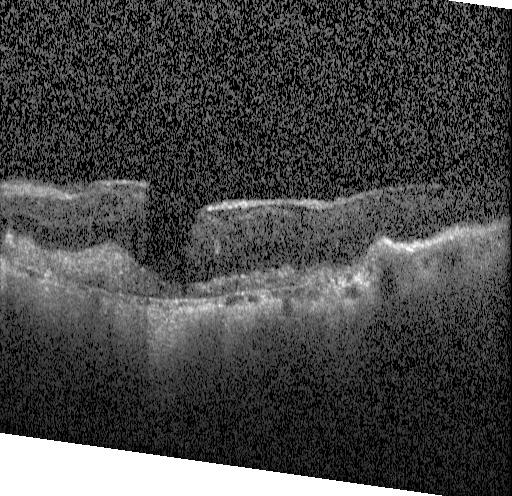
OCT B-scan · macular scan · spectral-domain optical coherence tomography · Heidelberg Spectralis.
Diagnosis: choroidal neovascularization.